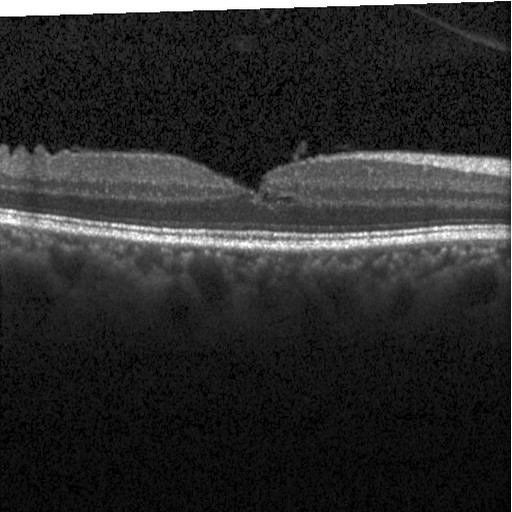

Acquired on a Heidelberg Spectralis; fovea-centered; optical coherence tomography B-scan.
Diagnosis: DME.